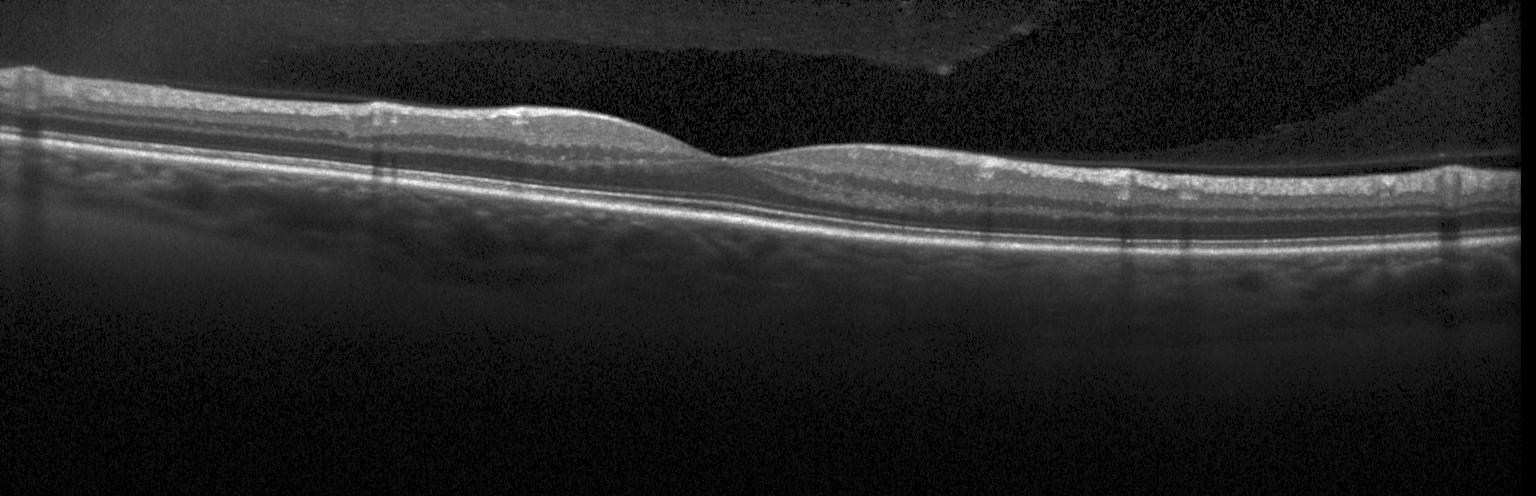 OCT finding: no evidence of choroidal neovascularization, diabetic macular edema, or drusen.